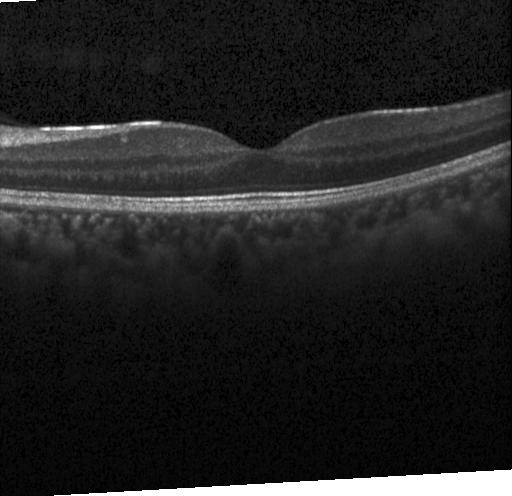

OCT line scan. Diagnosis: no choroidal neovascularization, no diabetic macular edema, and no drusen.